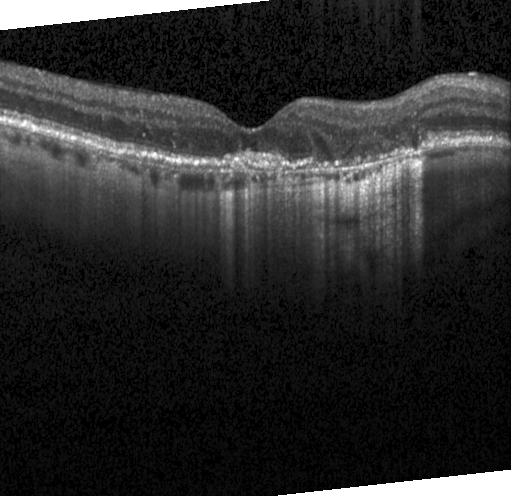

Retinal OCT B-scan, fovea-centered, instrument: Heidelberg Spectralis, spectral-domain OCT — Impression: a choroidal neovascular membrane.